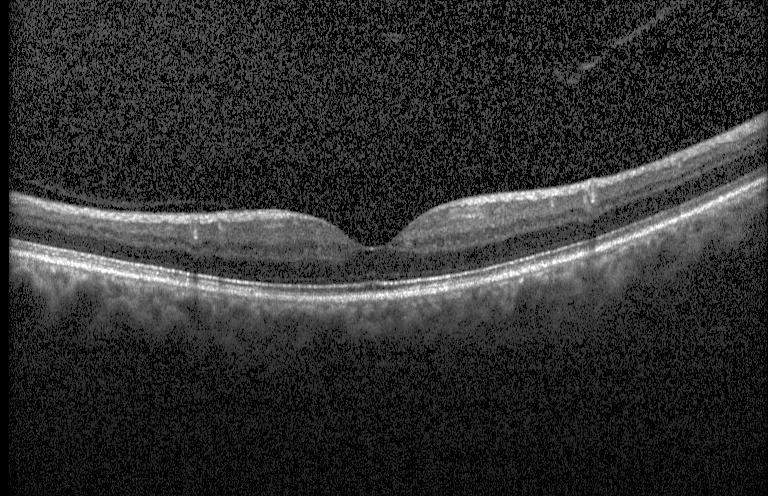
Centered on the fovea; SD-OCT; optical coherence tomography scan; Heidelberg Spectralis OCT system. OCT finding: no choroidal neovascularization, no diabetic macular edema, and no drusen.